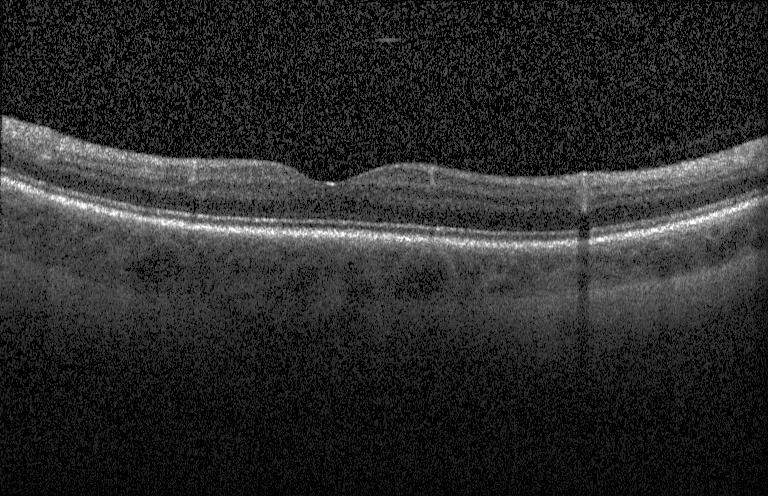 The scan shows no evidence of choroidal neovascularization, diabetic macular edema, or drusen.